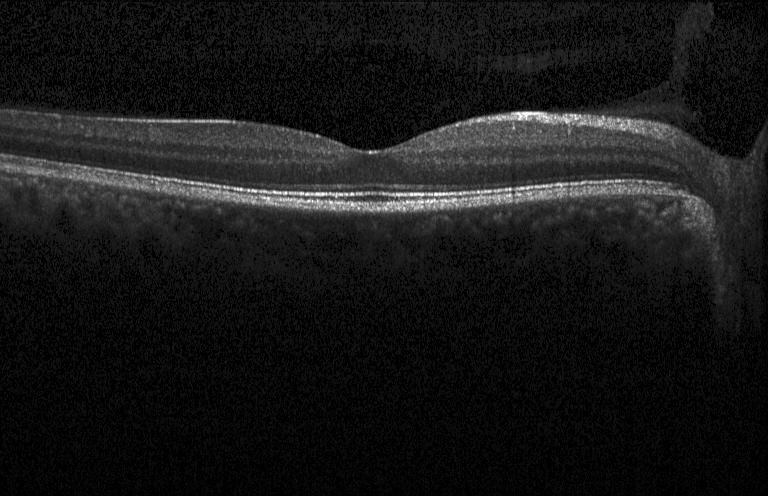

Optical coherence tomography B-scan — Impression: no choroidal neovascularization, no diabetic macular edema, and no drusen.